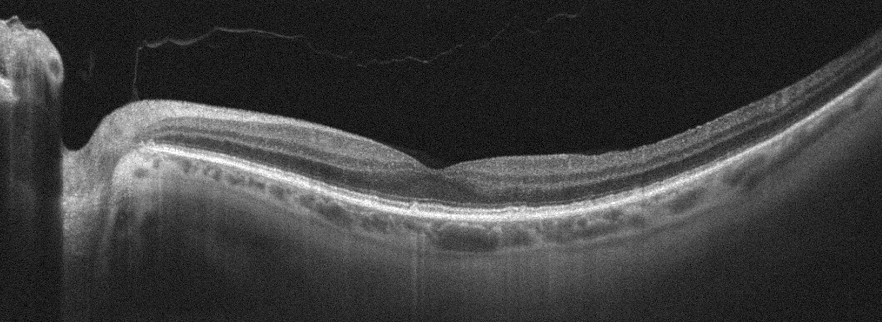 OCT B-scan; left eye. Diagnosis: age-related macular degeneration (AMD).